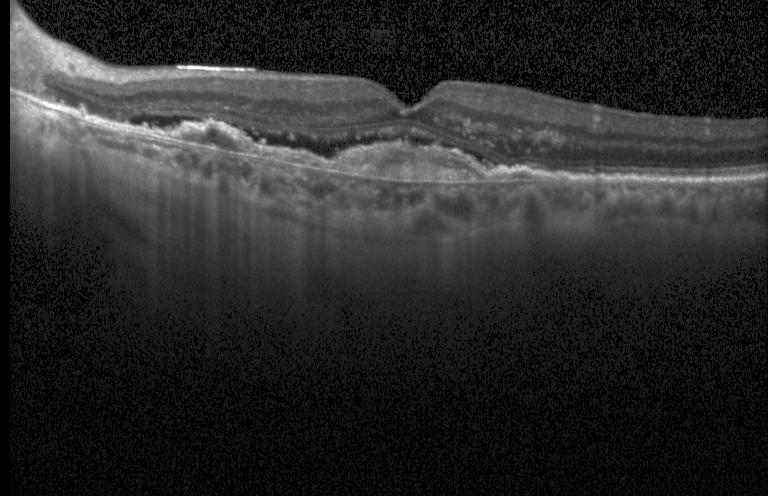

OCT B-scan showing a choroidal neovascular membrane.